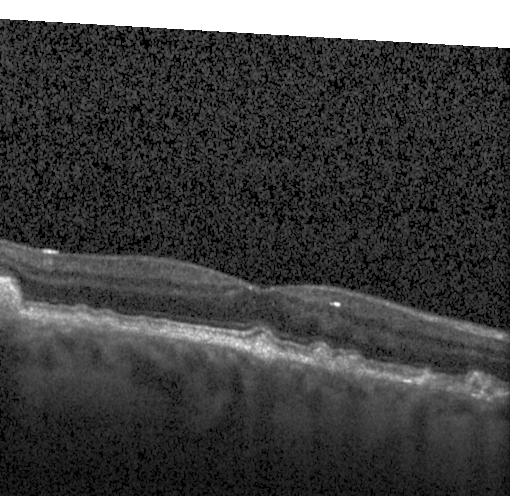
Impression: multiple drusen.